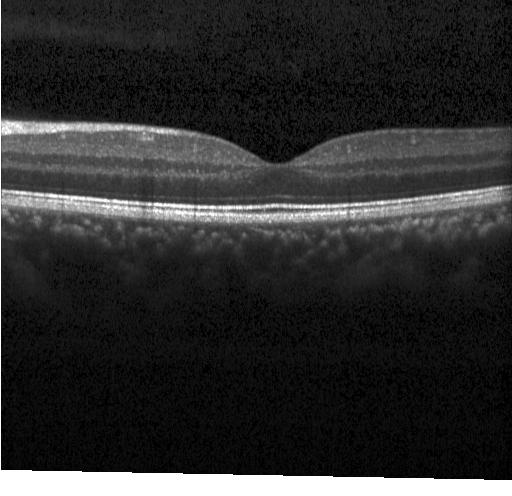 Dx: neither choroidal neovascularization, diabetic macular edema, nor drusen.